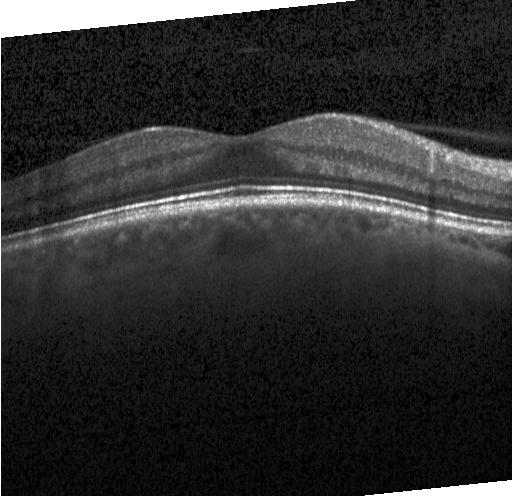

OCT line scan, Heidelberg Spectralis OCT system, spectral-domain optical coherence tomography. Impression: no choroidal neovascularization, no diabetic macular edema, and no drusen.